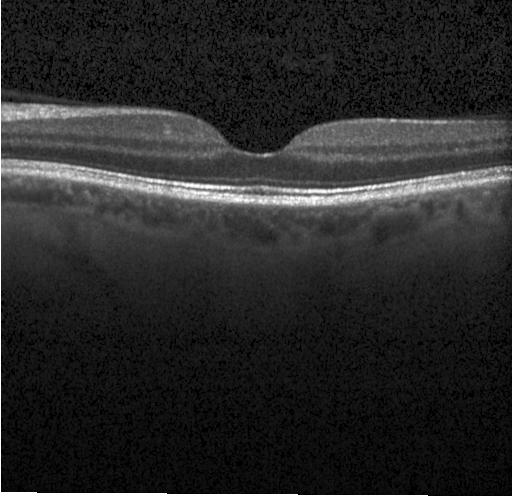

Retinal OCT cross-section. Spectral-domain OCT. Centered on the fovea. Acquired on a Heidelberg Spectralis
Diagnosis: no choroidal neovascularization, no diabetic macular edema, and no drusen.